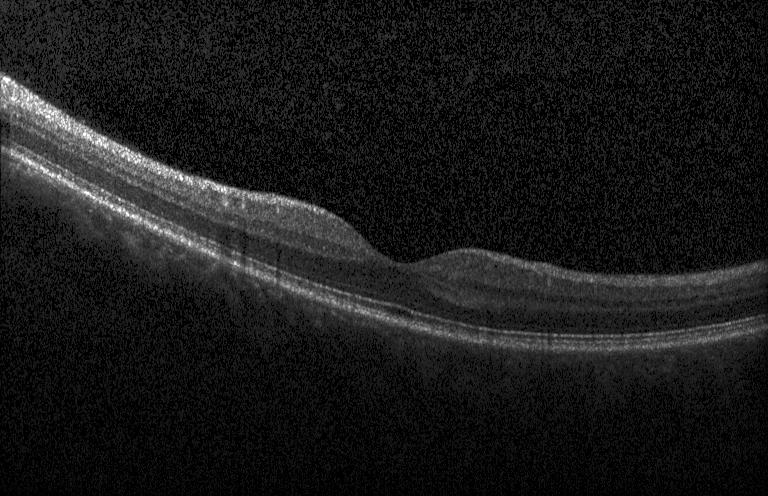
Through the macula. Retinal OCT cross-section
No evidence of choroidal neovascularization, diabetic macular edema, or drusen.